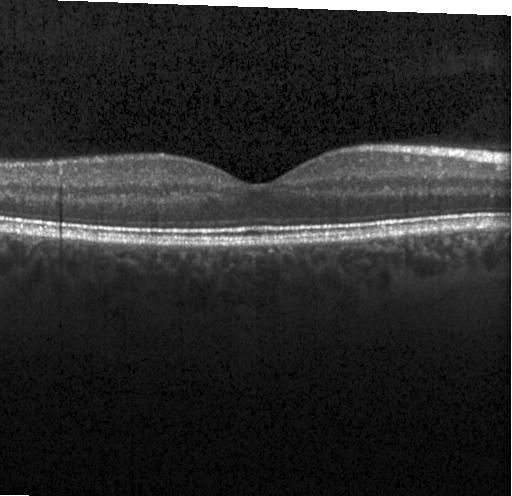
Optical coherence tomography scan.
This B-scan demonstrates no evidence of choroidal neovascularization, diabetic macular edema, or drusen.